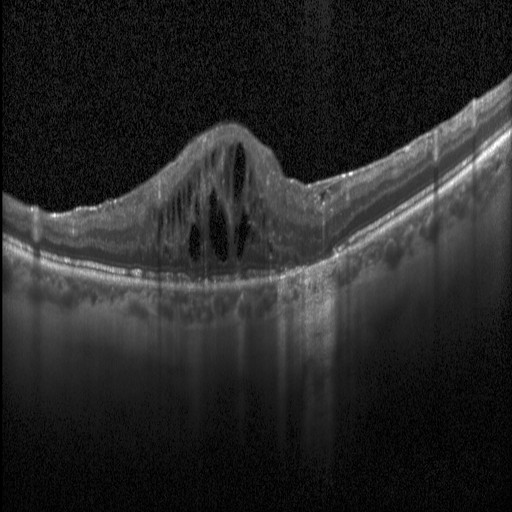

Retinal OCT cross-section
Finding: diabetic macular edema (DME).